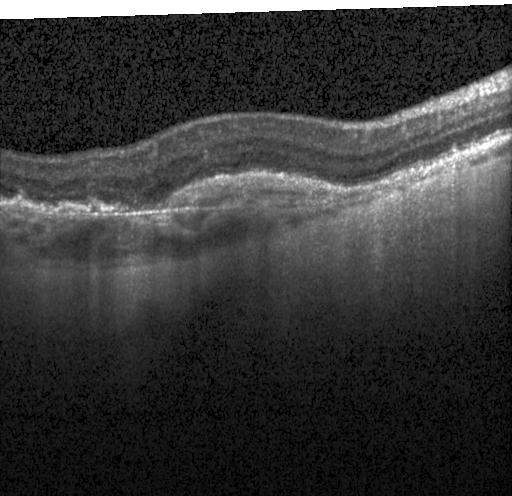
Diagnosis: a choroidal neovascular membrane.